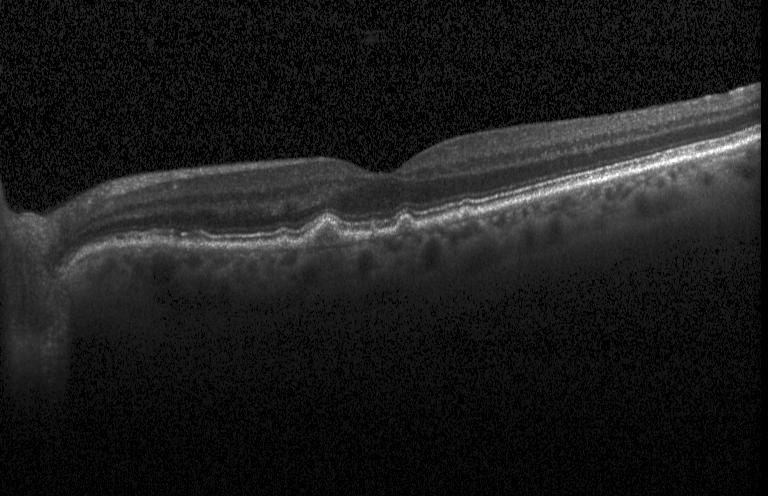

Acquired on a Heidelberg Spectralis, retinal OCT B-scan. Assessment: drusen.